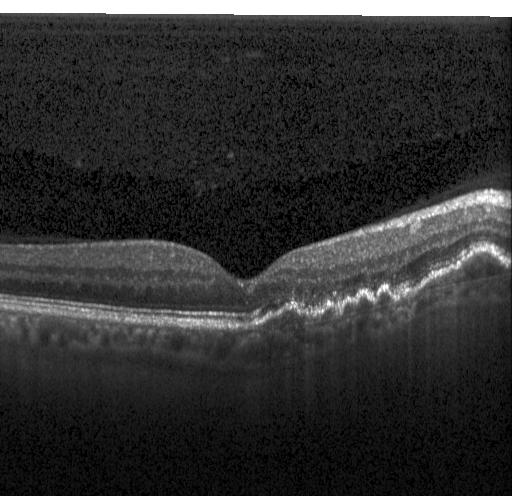
Retinal OCT cross-section
This B-scan demonstrates CNV.